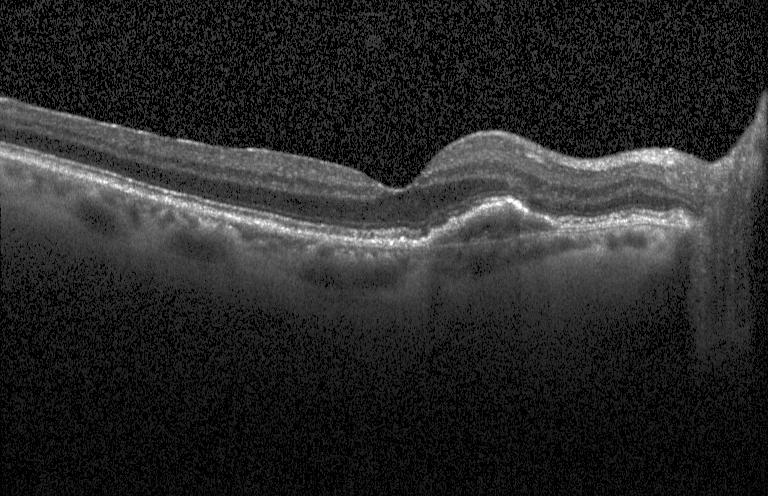
OCT B-scan — Impression: choroidal neovascularization.